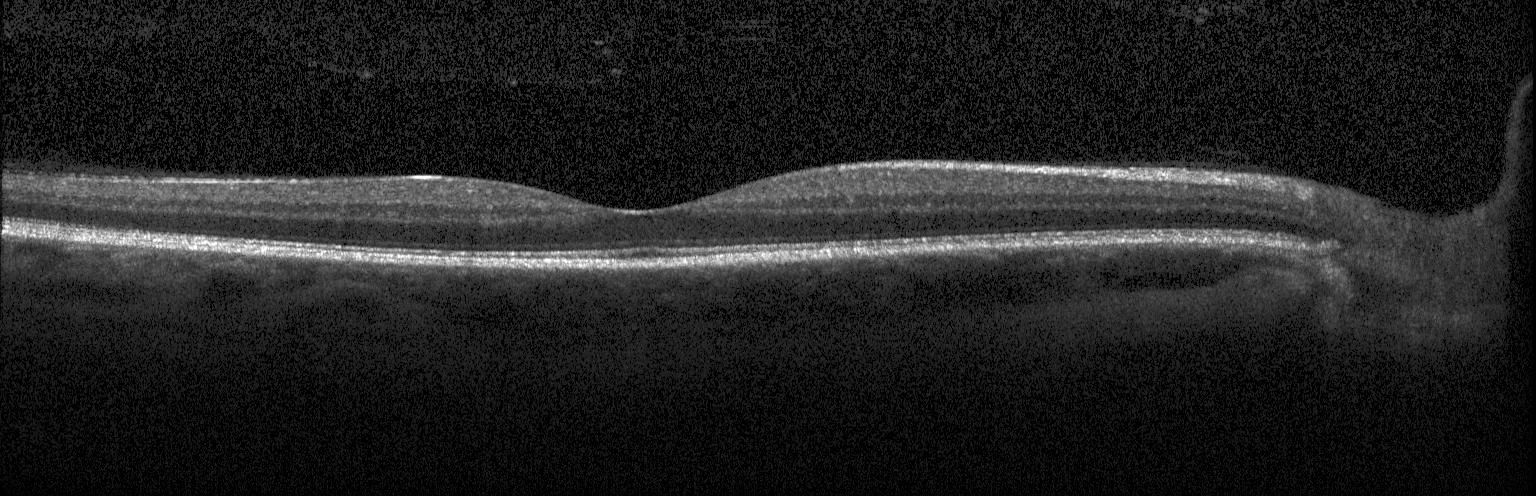 Optical coherence tomography B-scan
Impression: no choroidal neovascularization, diabetic macular edema, or drusen.